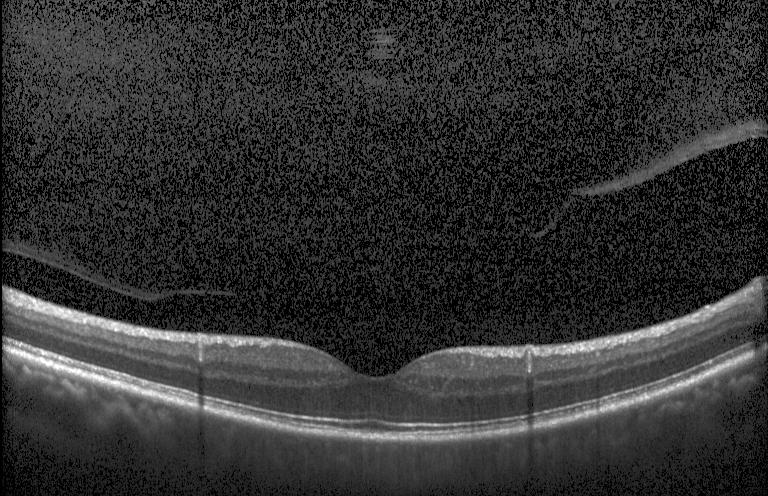

OCT line scan. Dx: no choroidal neovascularization, diabetic macular edema, or drusen.